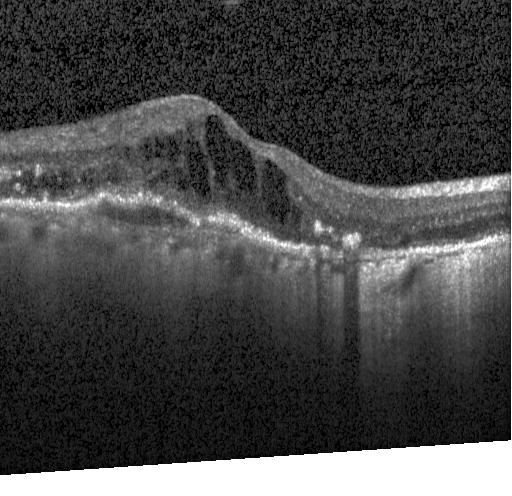

OCT B-scan · acquired on a Heidelberg Spectralis · spectral-domain OCT.
Assessment: CNV.